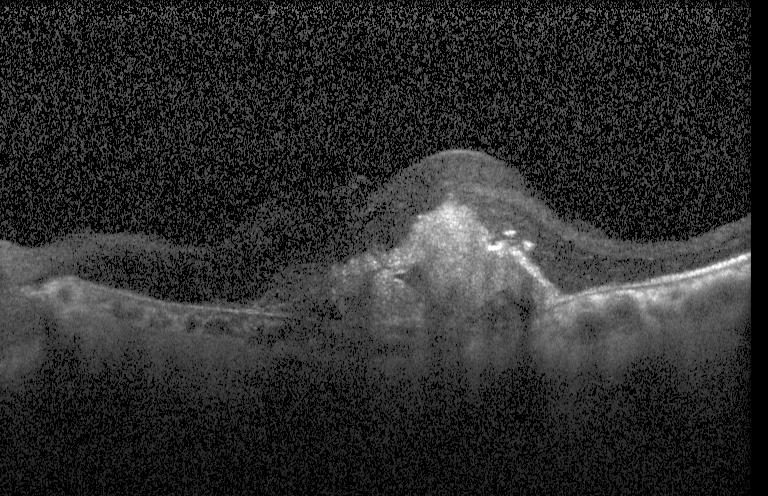 Macular scan · Heidelberg Spectralis · optical coherence tomography B-scan · spectral-domain OCT
Finding: a choroidal neovascular membrane.